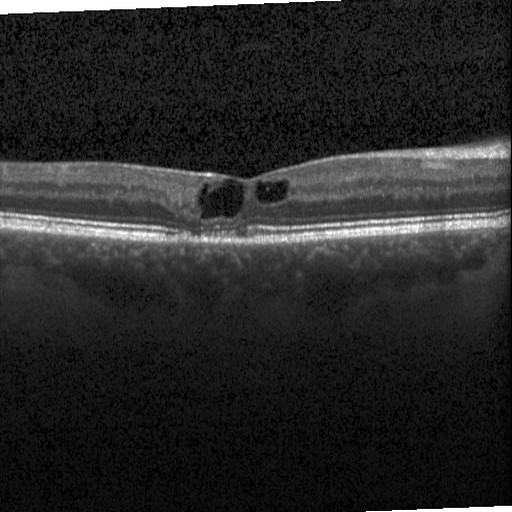
Macular scan, retinal OCT B-scan
Diagnosis: diabetic macular edema (DME).